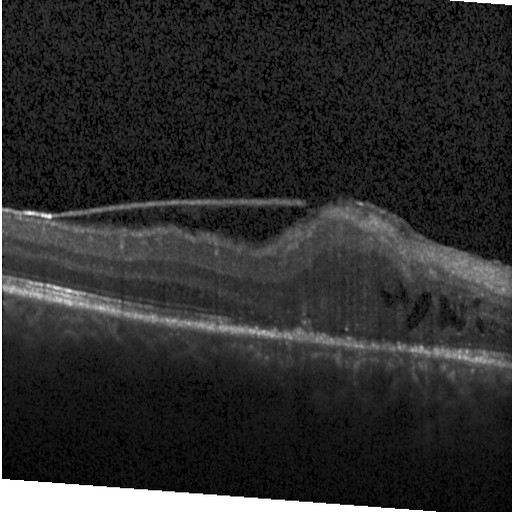
Retinal OCT B-scan. Heidelberg Spectralis. SD-OCT. Fovea-centered — This B-scan demonstrates diabetic macular edema.